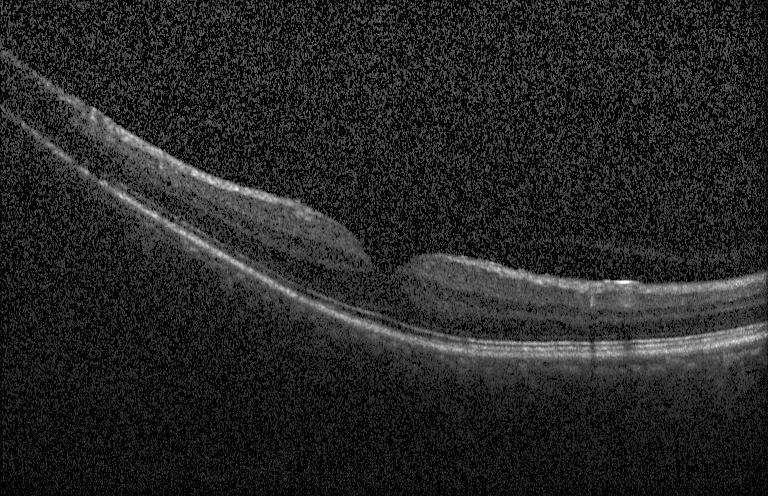

Heidelberg Spectralis OCT system. Retinal OCT cross-section.
Impression: no choroidal neovascularization, no diabetic macular edema, and no drusen.